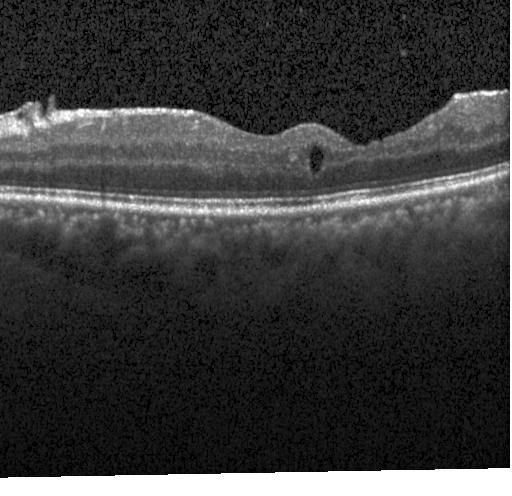 Optical coherence tomography scan — Diagnosis: DME.